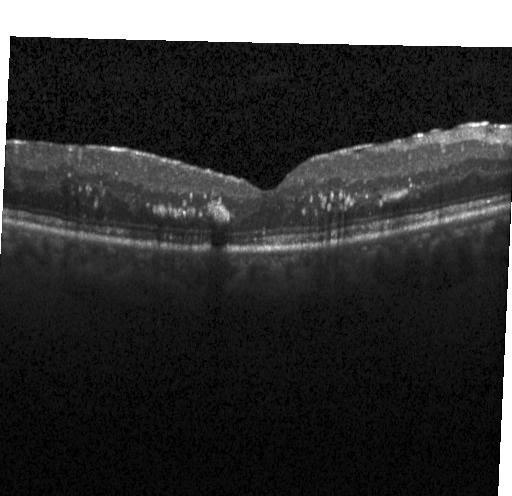

Finding: diabetic macular edema.